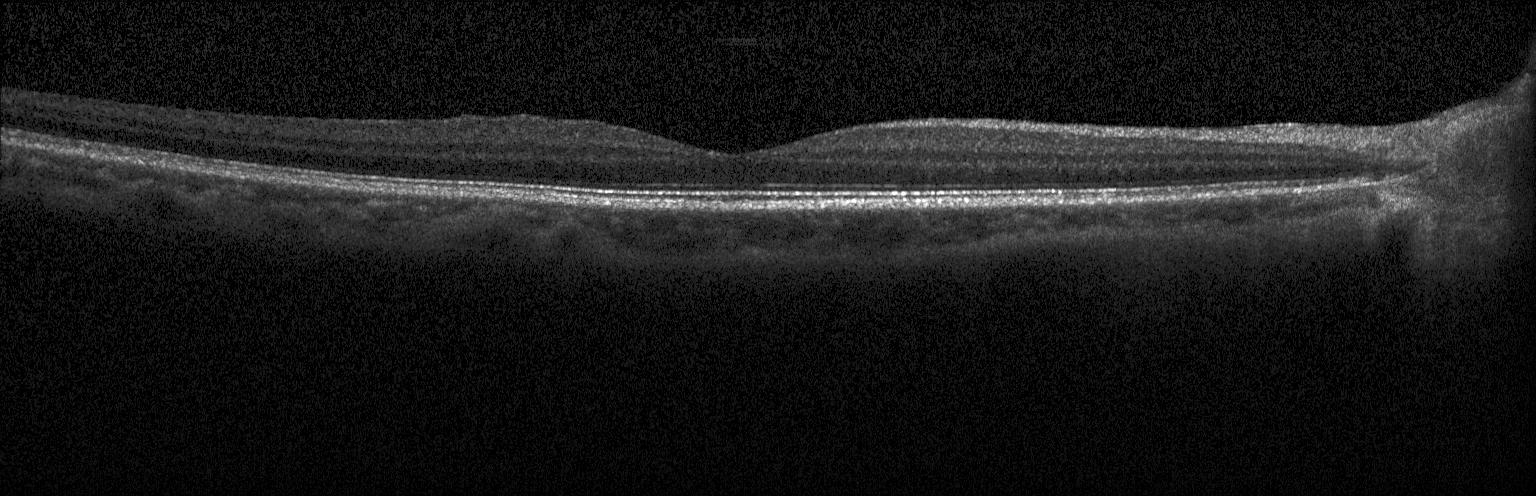

Retinal OCT cross-section · horizontal scan through the fovea · Heidelberg Spectralis OCT system · spectral-domain OCT — OCT finding: no CNV, DME, or drusen.